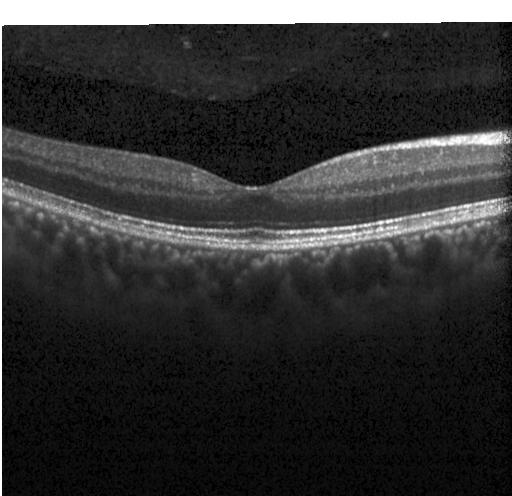

Optical coherence tomography B-scan
Impression: neither choroidal neovascularization, diabetic macular edema, nor drusen.